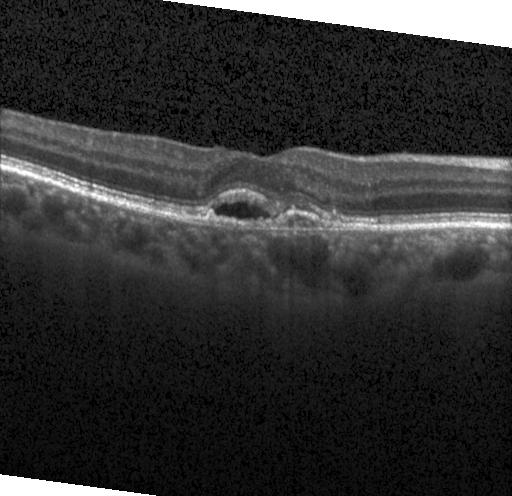 Finding: a choroidal neovascular membrane.